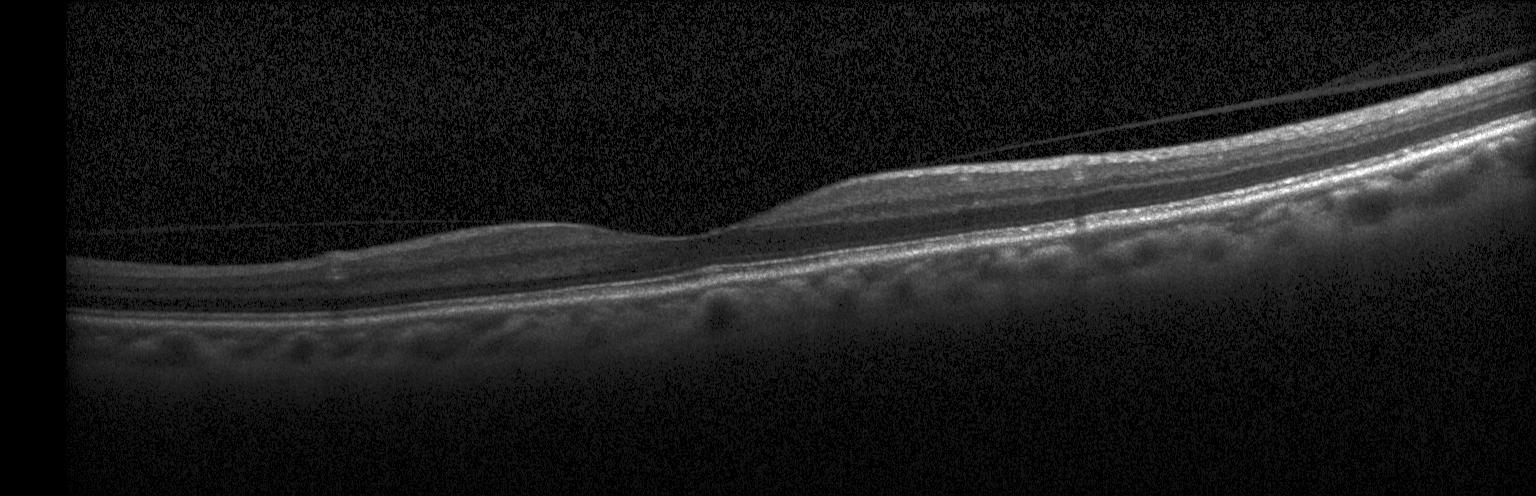

Optical coherence tomography B-scan; macular scan. No choroidal neovascularization, no diabetic macular edema, and no drusen.